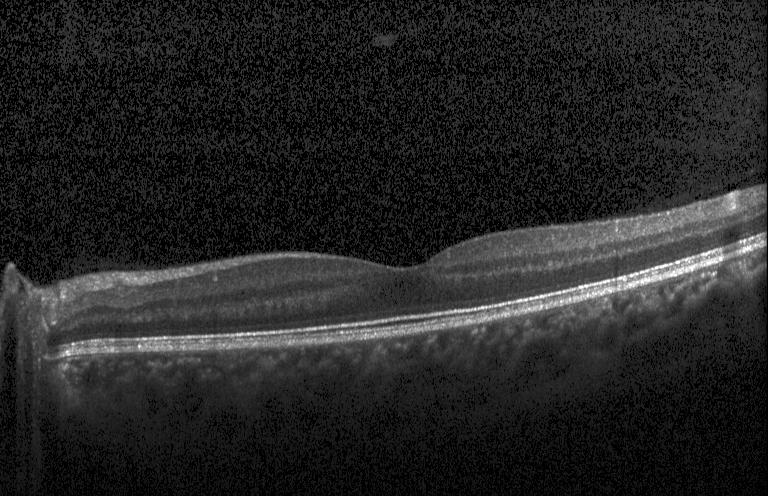 OCT finding: no choroidal neovascularization, no diabetic macular edema, and no drusen.